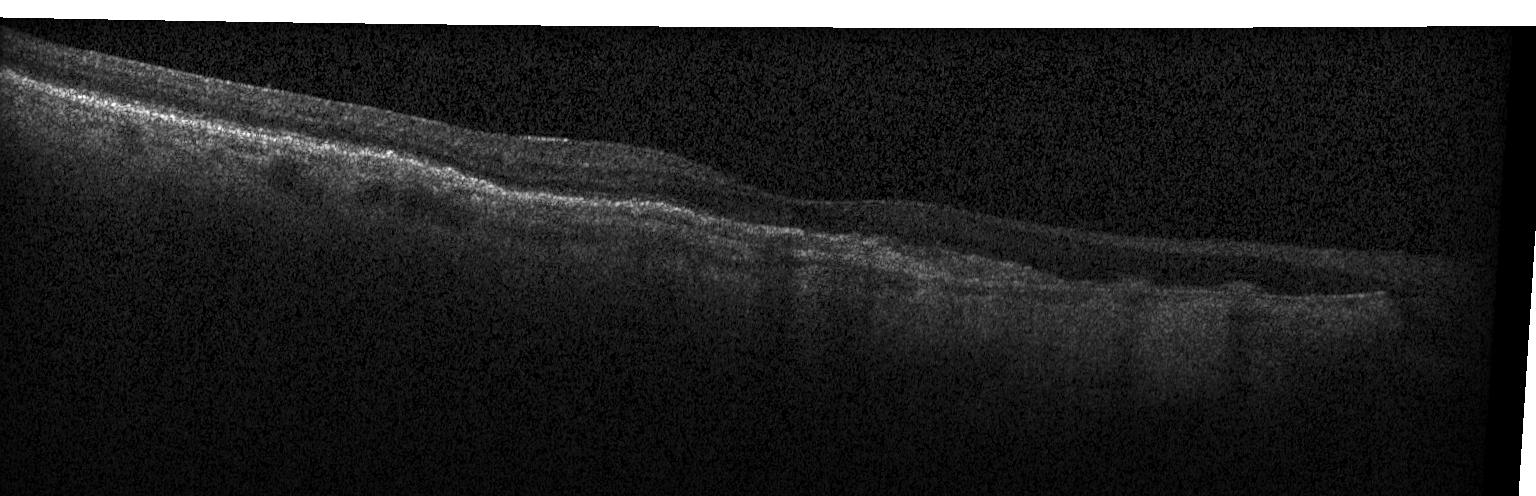 OCT line scan · macular scan.
Finding: choroidal neovascularization.